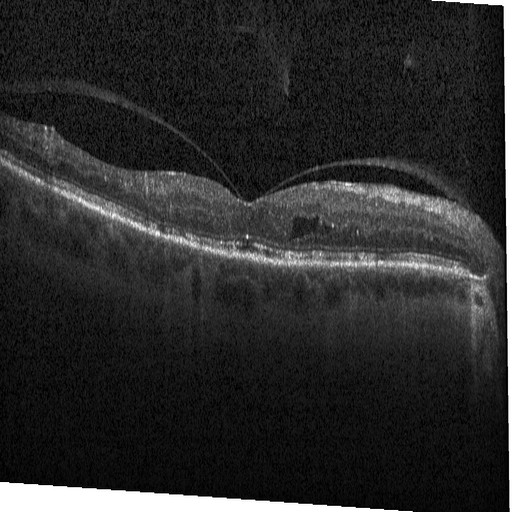

Retinal OCT cross-section — Finding: diabetic macular edema.